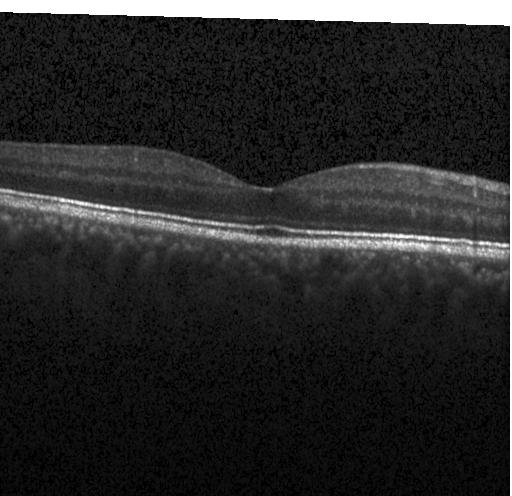

Macular OCT demonstrating no evidence of CNV, DME, or drusen.